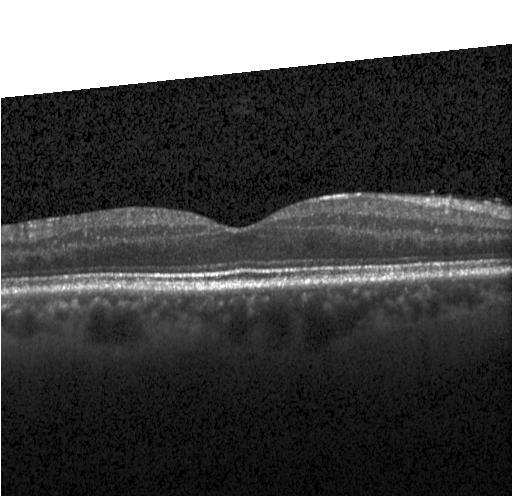
Macular OCT: no choroidal neovascularization, diabetic macular edema, or drusen.